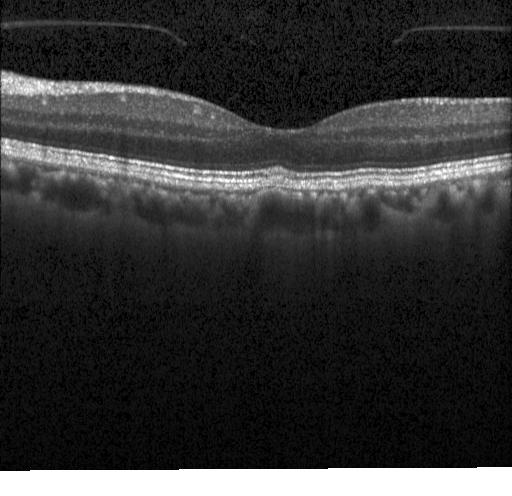 Optical coherence tomography scan · macular scan · Heidelberg Spectralis OCT system · spectral-domain OCT.
No CNV, no DME, and no drusen.